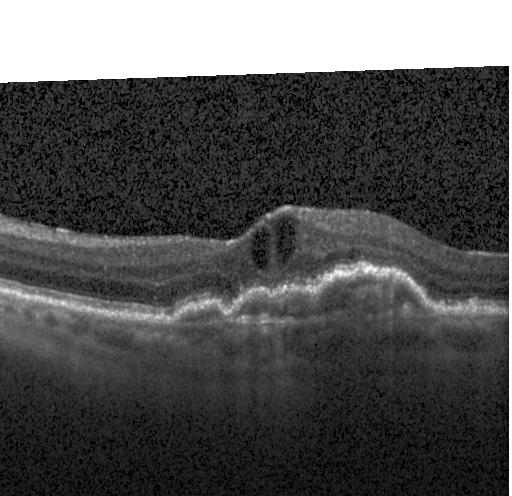 Instrument: Heidelberg Spectralis; macular scan; retinal OCT cross-section.
Finding: choroidal neovascularization (CNV).